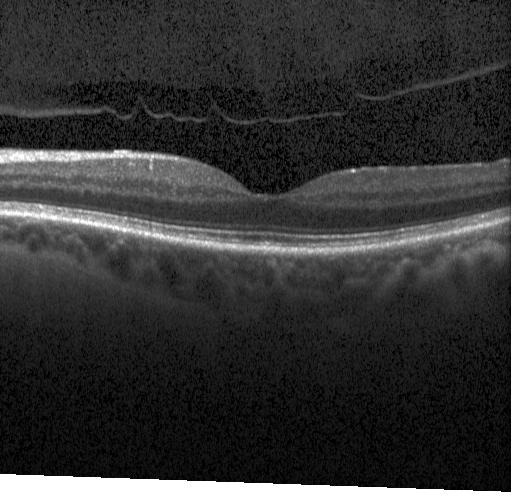
Diagnosis: no choroidal neovascularization, no diabetic macular edema, and no drusen.